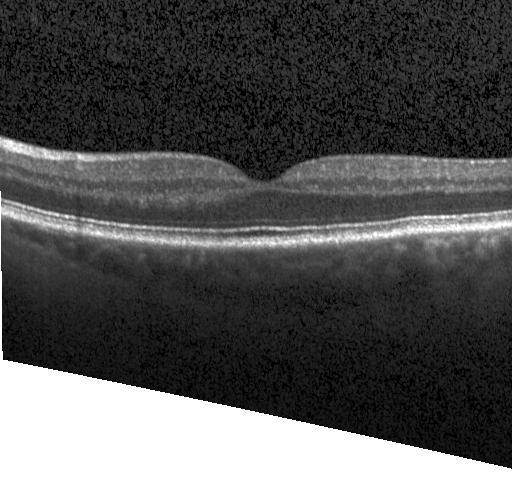
SD-OCT. Optical coherence tomography scan. Centered on the fovea. Instrument: Heidelberg Spectralis.
The scan shows no CNV, no DME, and no drusen.